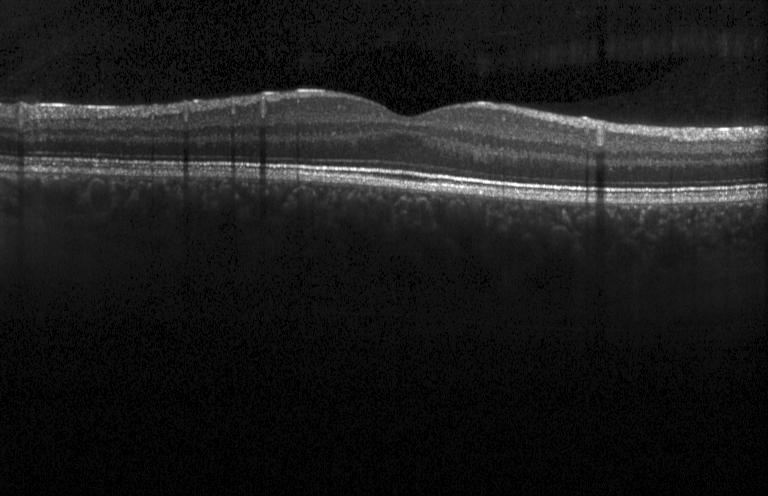

Instrument: Heidelberg Spectralis, optical coherence tomography B-scan — Macular OCT: no CNV, no DME, and no drusen.